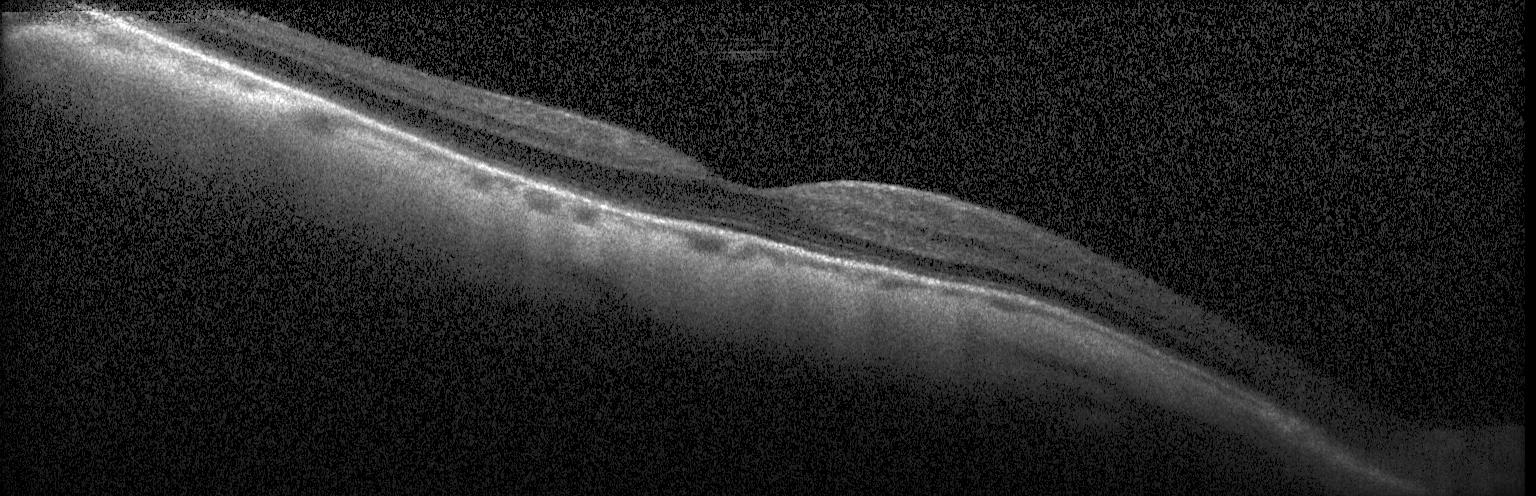

Through the macula. Retinal OCT cross-section. Diagnosis: neither CNV, DME, nor drusen.